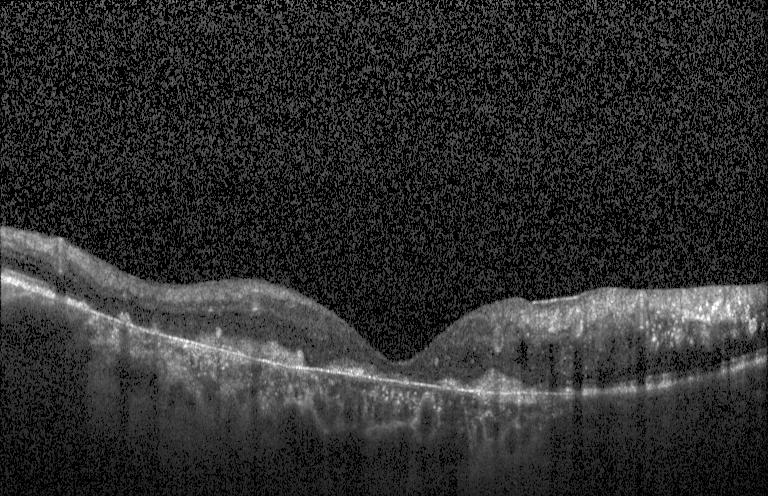 Diagnosis: choroidal neovascularization.